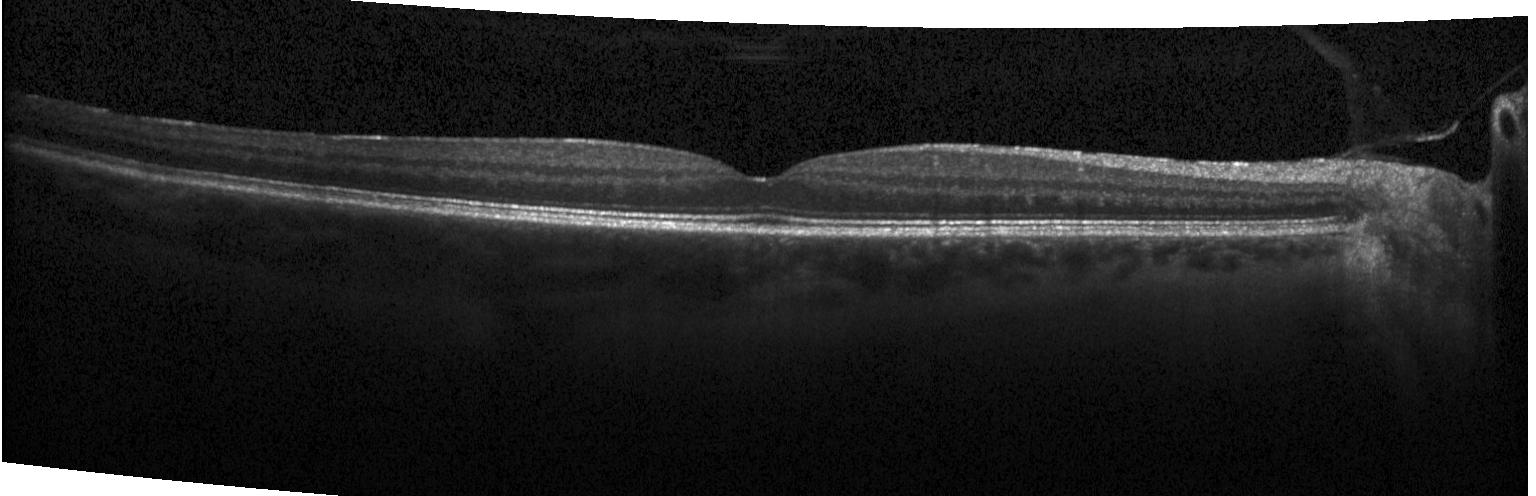
Acquired on a Heidelberg Spectralis; retinal OCT cross-section.
Diagnosis: no choroidal neovascularization, diabetic macular edema, or drusen.